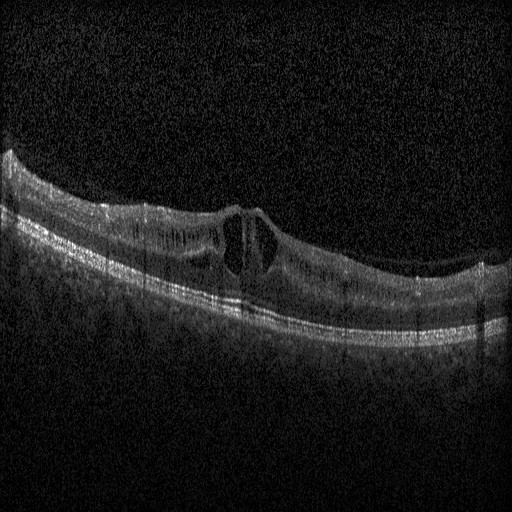 Retinal OCT B-scan
Diagnosis: diabetic macular edema.